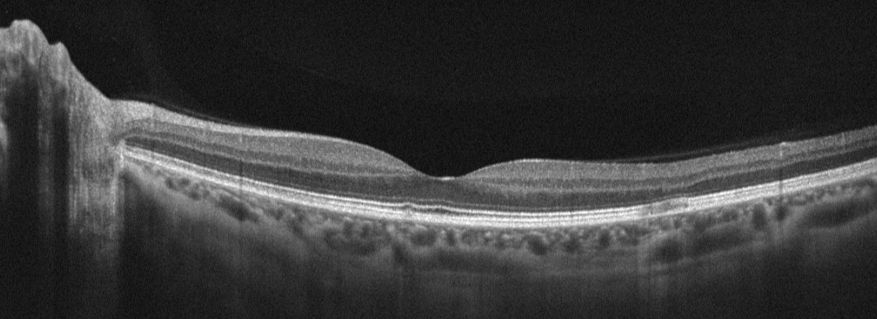

Diagnosis: absence of AMD, DME, ERM, RAO, RVO, and vitreomacular interface disease.